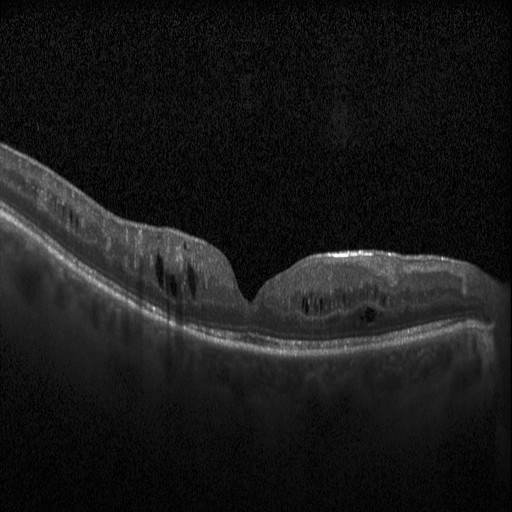
OCT finding: DME.